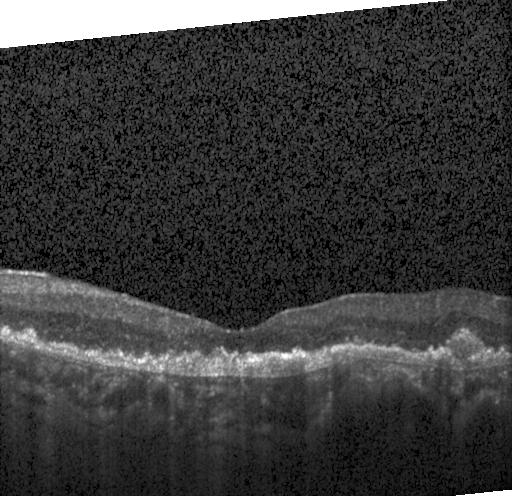 Retinal OCT B-scan · SD-OCT — Assessment: a choroidal neovascular membrane.